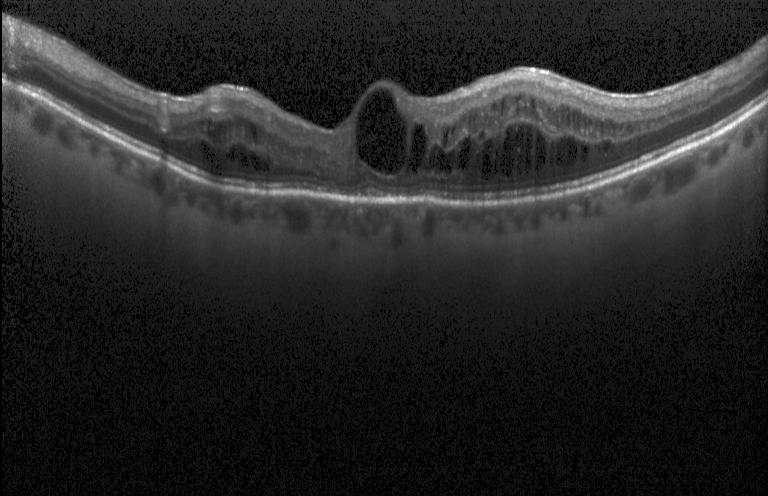
The scan shows DME.